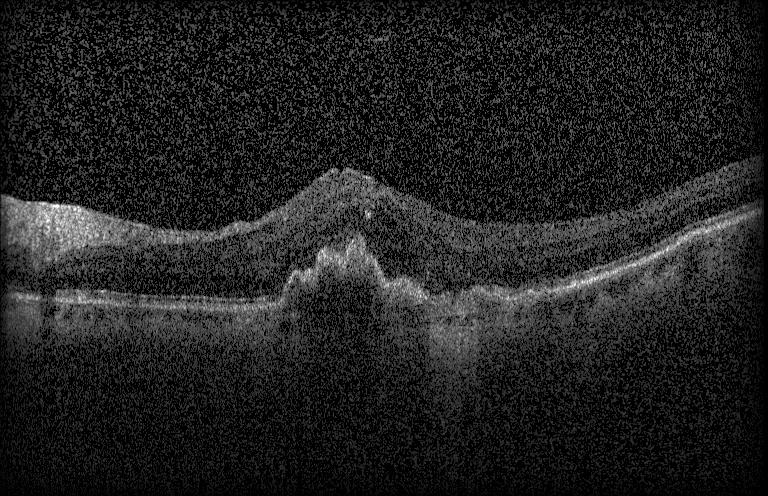
Impression: a choroidal neovascular membrane.